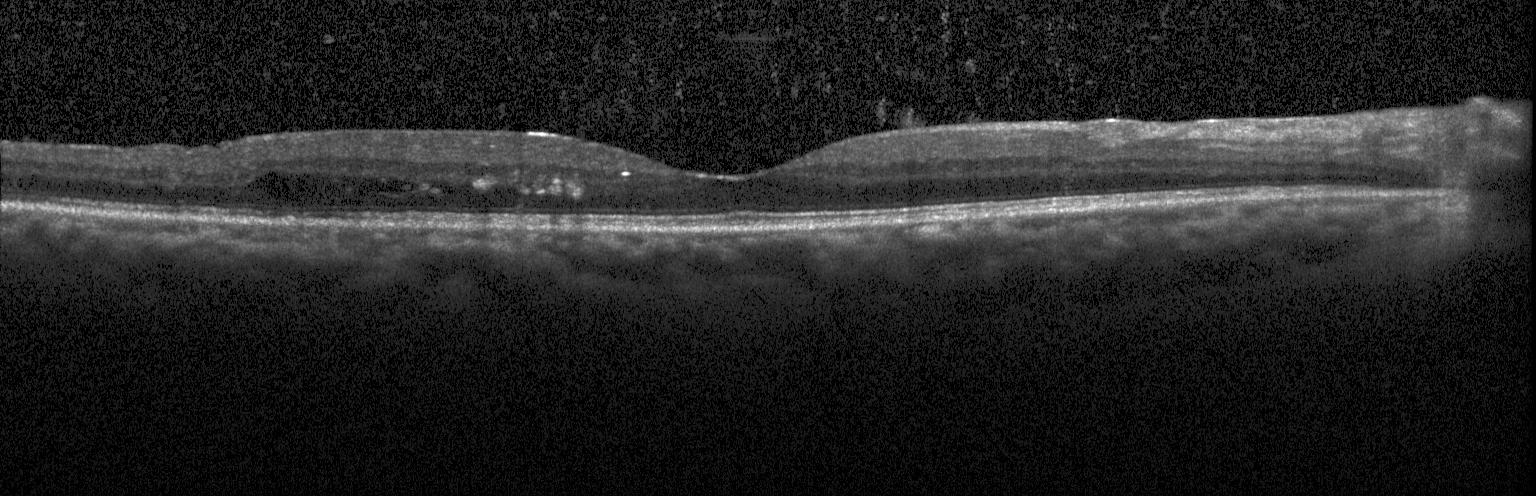

Retinal OCT B-scan; Heidelberg Spectralis.
OCT finding: diabetic macular edema (DME).